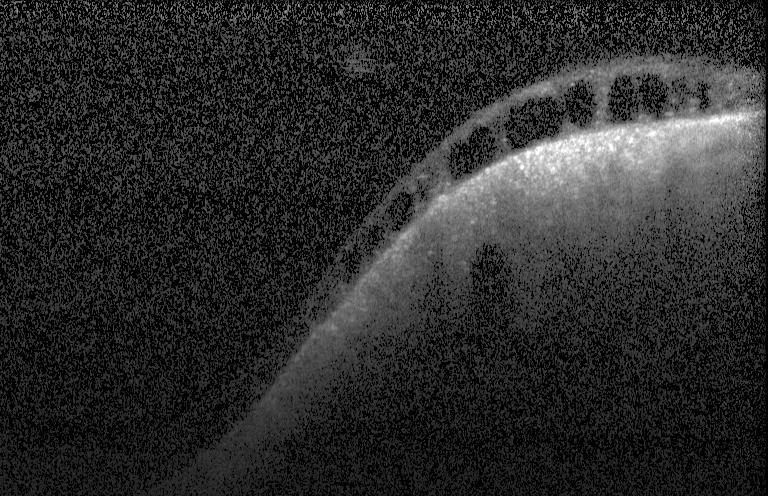

Macular OCT demonstrating DME.